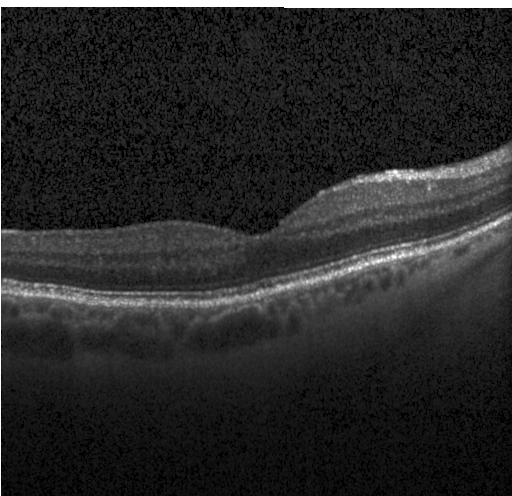
Diagnosis: no choroidal neovascularization, diabetic macular edema, or drusen.